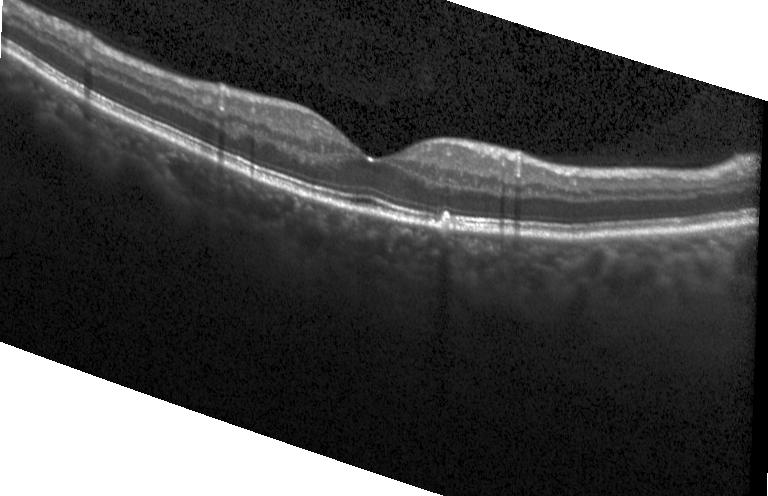 OCT line scan. Dx: sub-RPE drusenoid deposits.